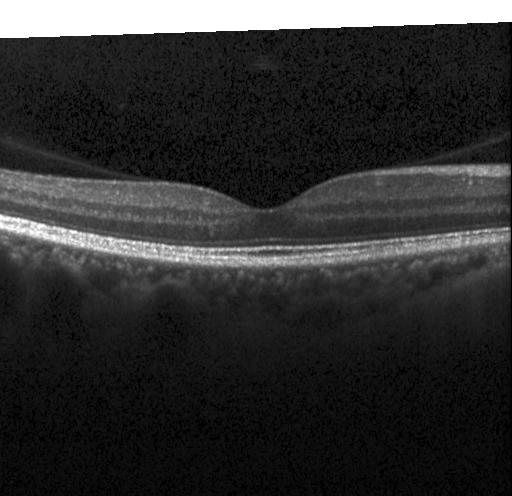
OCT finding: no choroidal neovascularization, no diabetic macular edema, and no drusen.